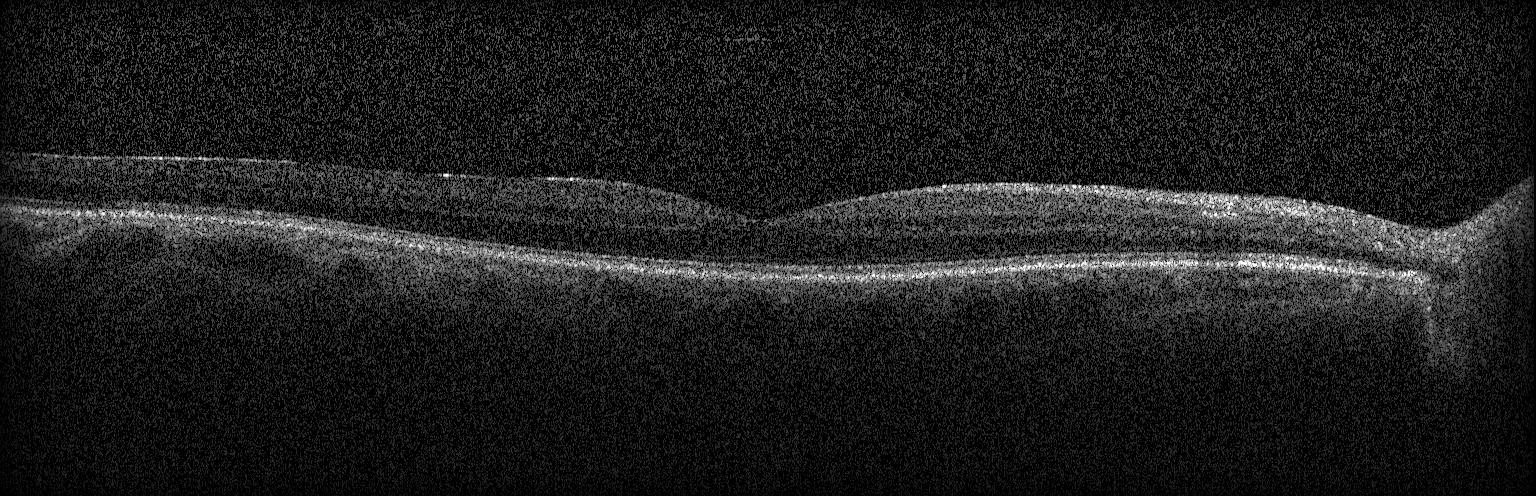 OCT line scan
OCT finding: no choroidal neovascularization, diabetic macular edema, or drusen.